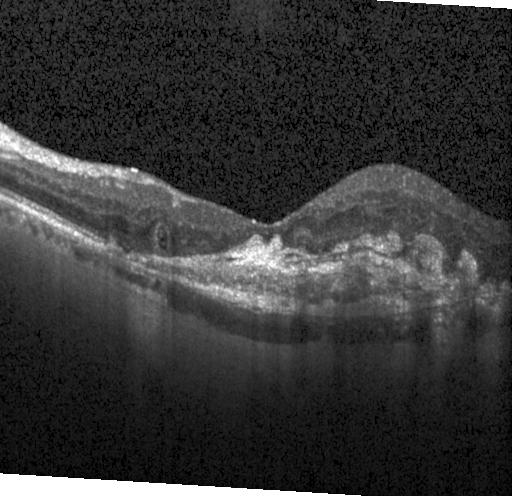
Macular OCT demonstrating choroidal neovascularization (CNV).